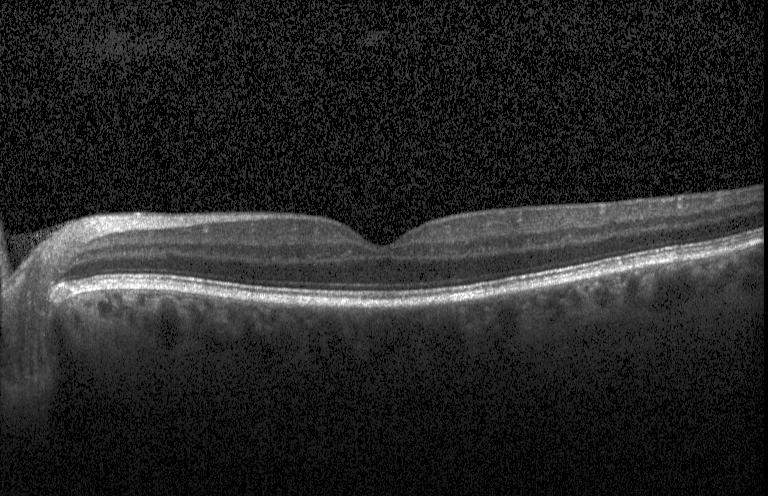

Acquired on a Heidelberg Spectralis, spectral-domain OCT, retinal OCT cross-section — Diagnosis: no evidence of choroidal neovascularization, diabetic macular edema, or drusen.